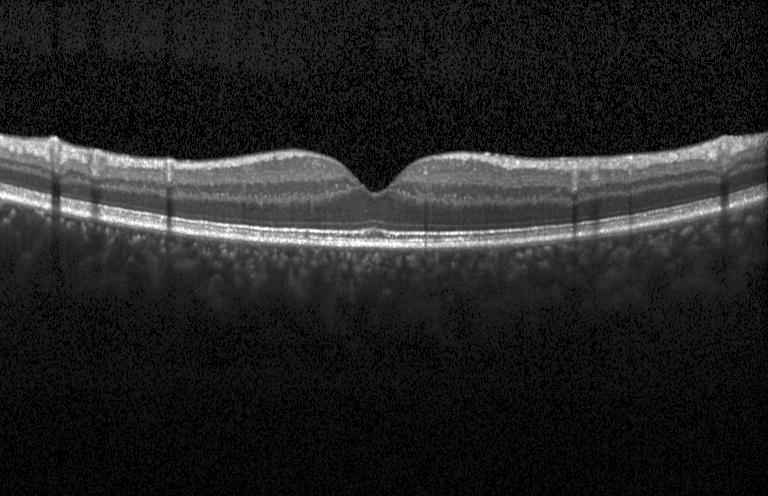

Diagnosis: no evidence of choroidal neovascularization, diabetic macular edema, or drusen.